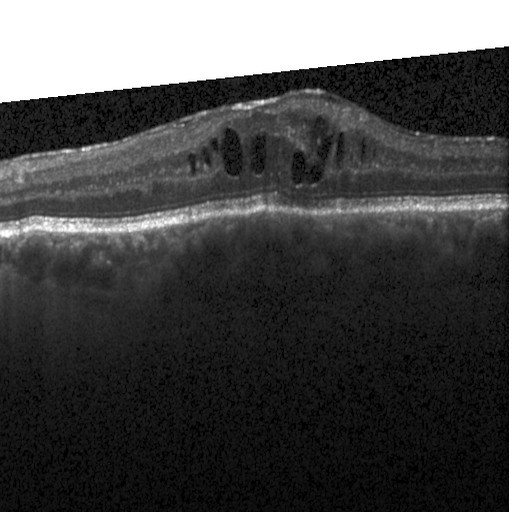
Optical coherence tomography scan. Fovea-centered. SD-OCT. This B-scan demonstrates DME.